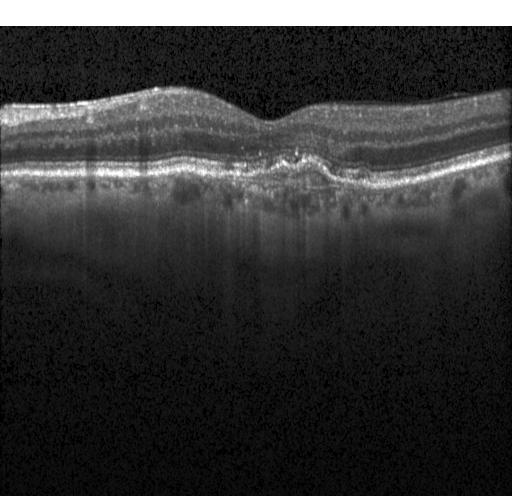
Heidelberg Spectralis · SD-OCT · retinal OCT B-scan · fovea-centered
OCT finding: a choroidal neovascular membrane.